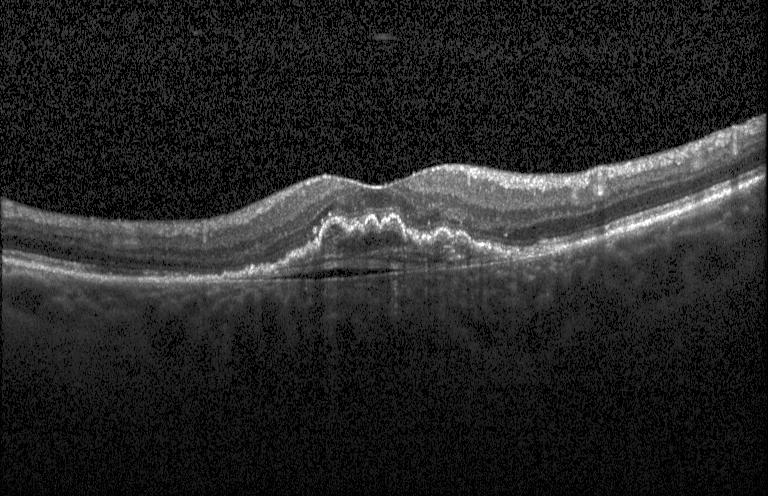
OCT B-scan showing a choroidal neovascular membrane.